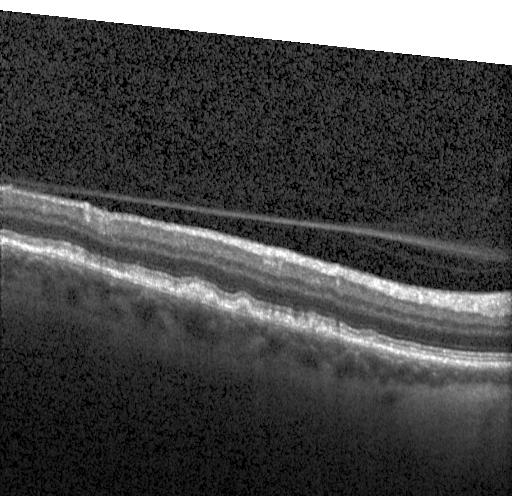

Finding: sub-RPE drusenoid deposits.